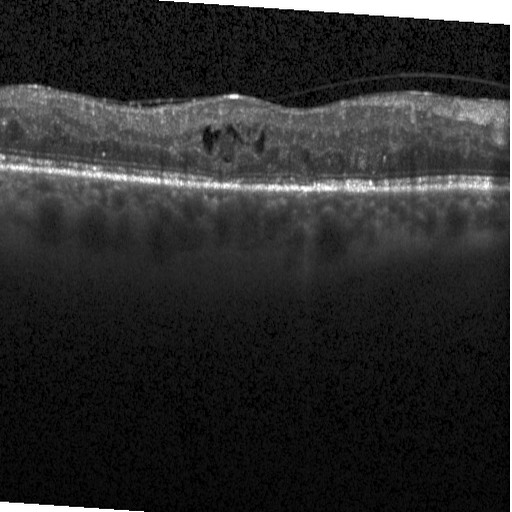
Spectral-domain optical coherence tomography · macular scan · optical coherence tomography B-scan — This B-scan demonstrates diabetic macular edema.